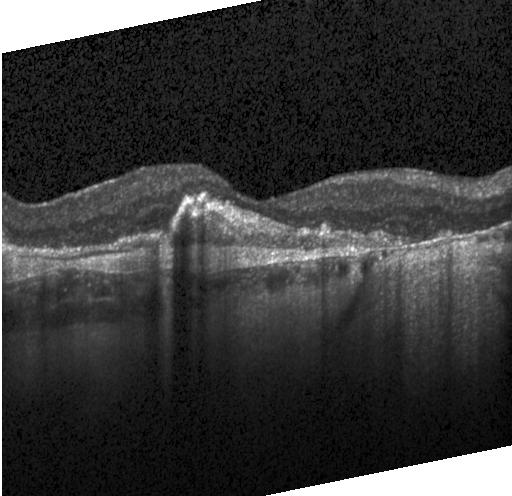 Diagnosis: CNV.